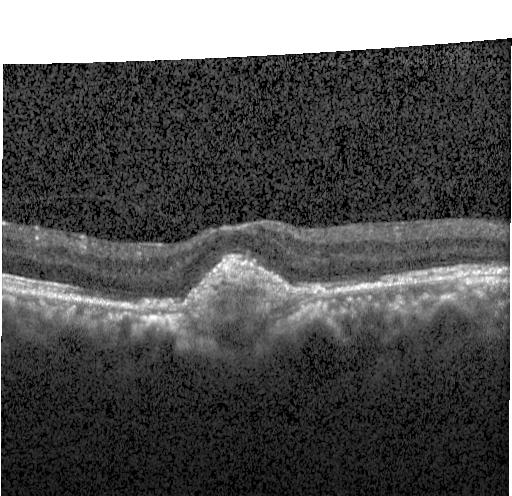 Heidelberg Spectralis OCT system · retinal OCT B-scan · SD-OCT.
A choroidal neovascular membrane.